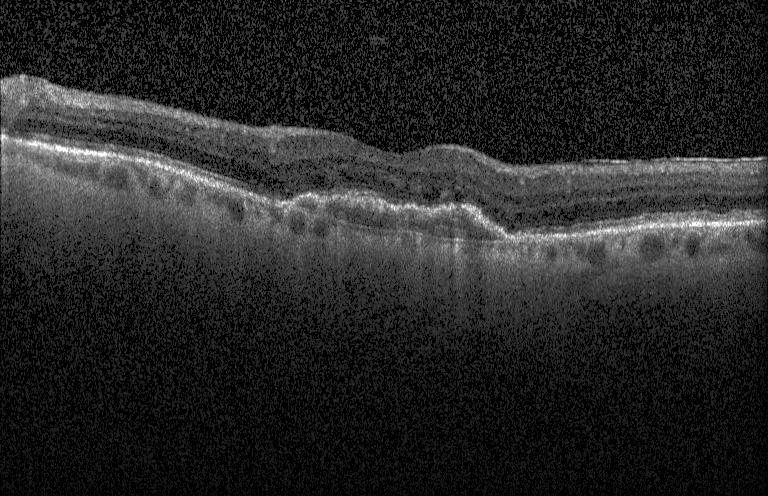 Acquired on a Heidelberg Spectralis, fovea-centered, spectral-domain optical coherence tomography, OCT B-scan. Assessment: choroidal neovascularization (CNV).